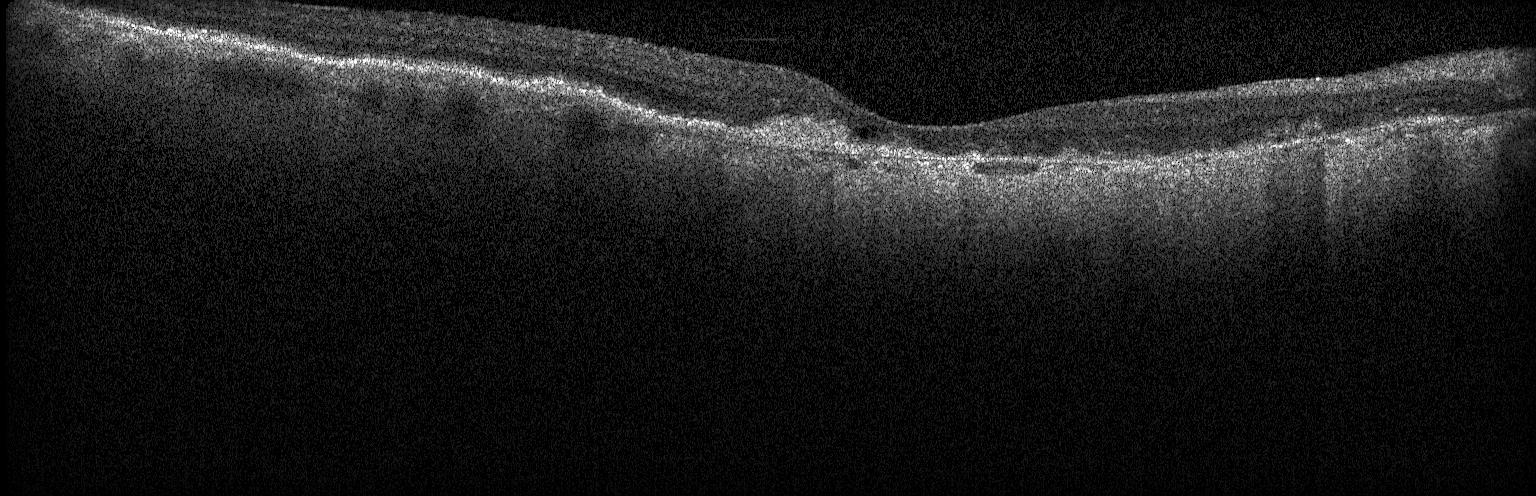 Optical coherence tomography B-scan, through the macula, SD-OCT — This B-scan demonstrates choroidal neovascularization.